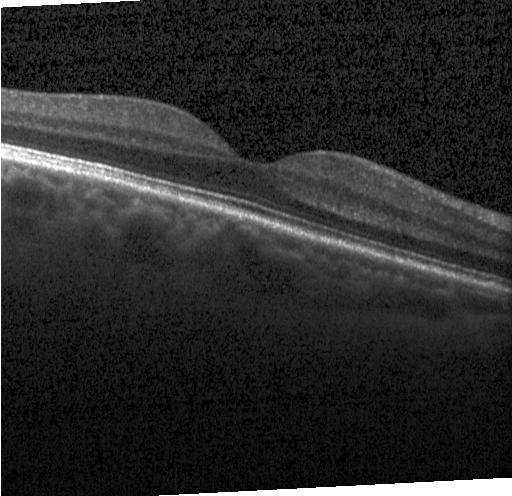

The scan shows no choroidal neovascularization, no diabetic macular edema, and no drusen.